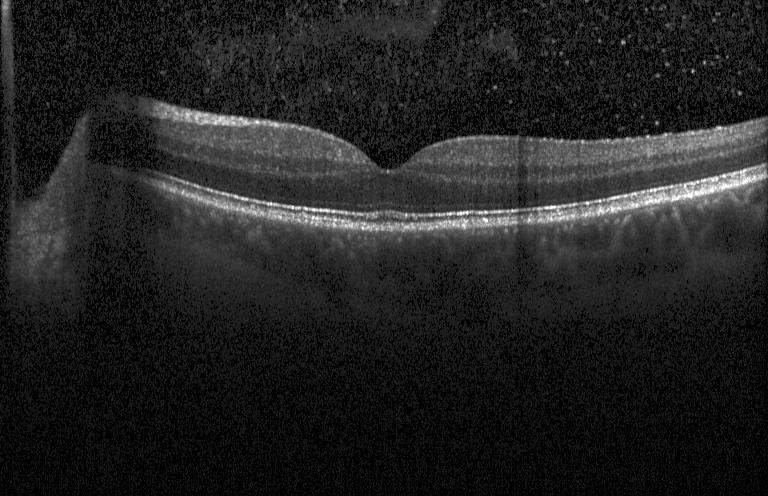
Retinal OCT cross-section; SD-OCT.
Impression: no CNV, no DME, and no drusen.